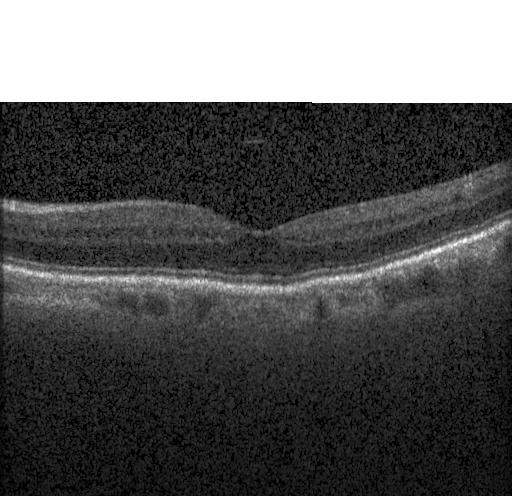 Diagnosis: no choroidal neovascularization, no diabetic macular edema, and no drusen.